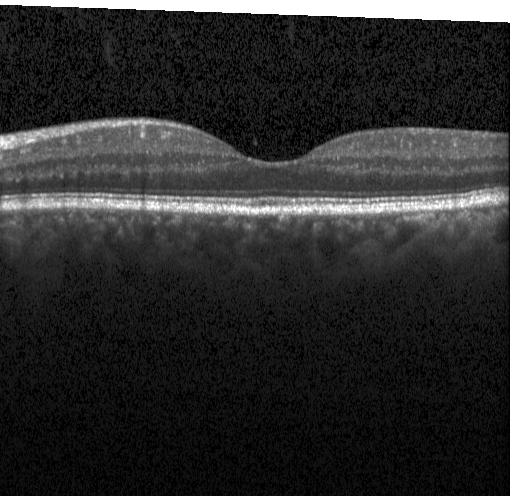 OCT finding: neither choroidal neovascularization, diabetic macular edema, nor drusen.